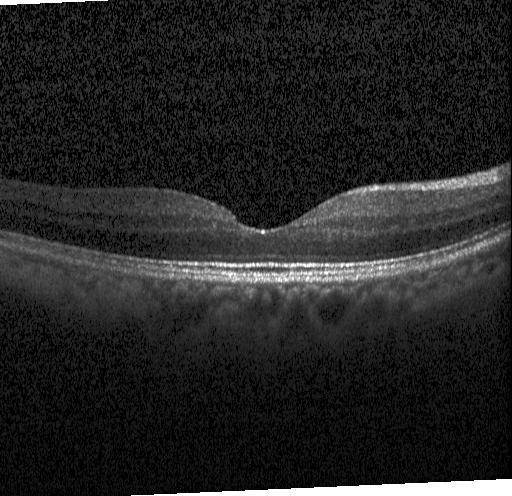
Horizontal scan through the fovea, retinal OCT cross-section, spectral-domain OCT — Finding: no CNV, DME, or drusen.